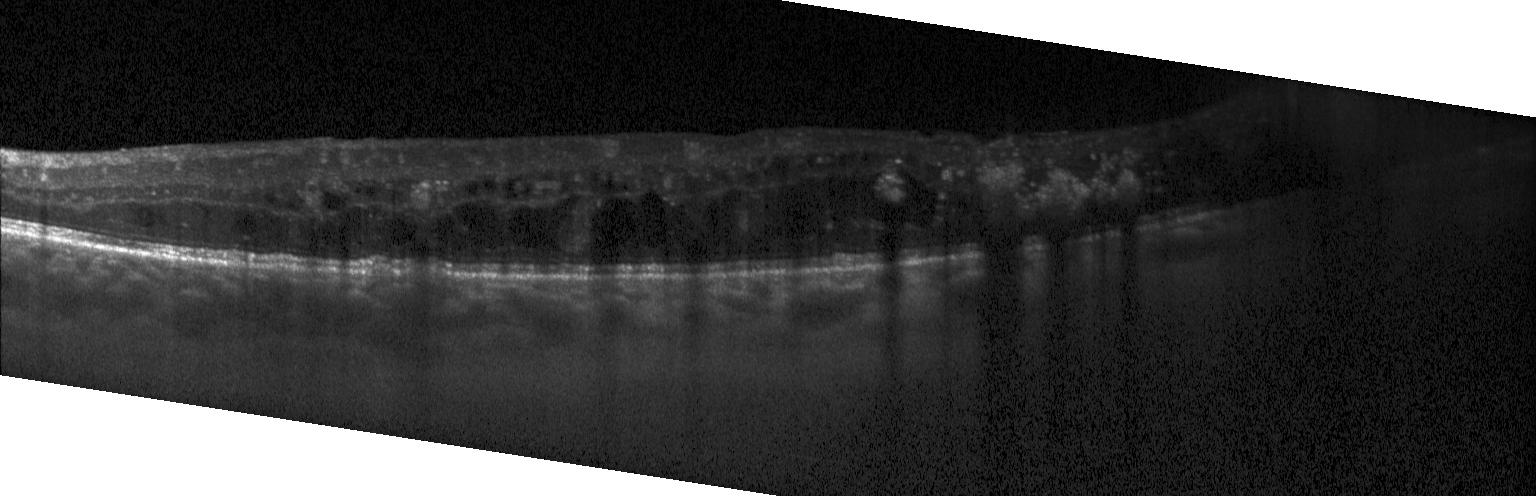 SD-OCT · retinal OCT cross-section · centered on the fovea
The scan shows diabetic macular edema.